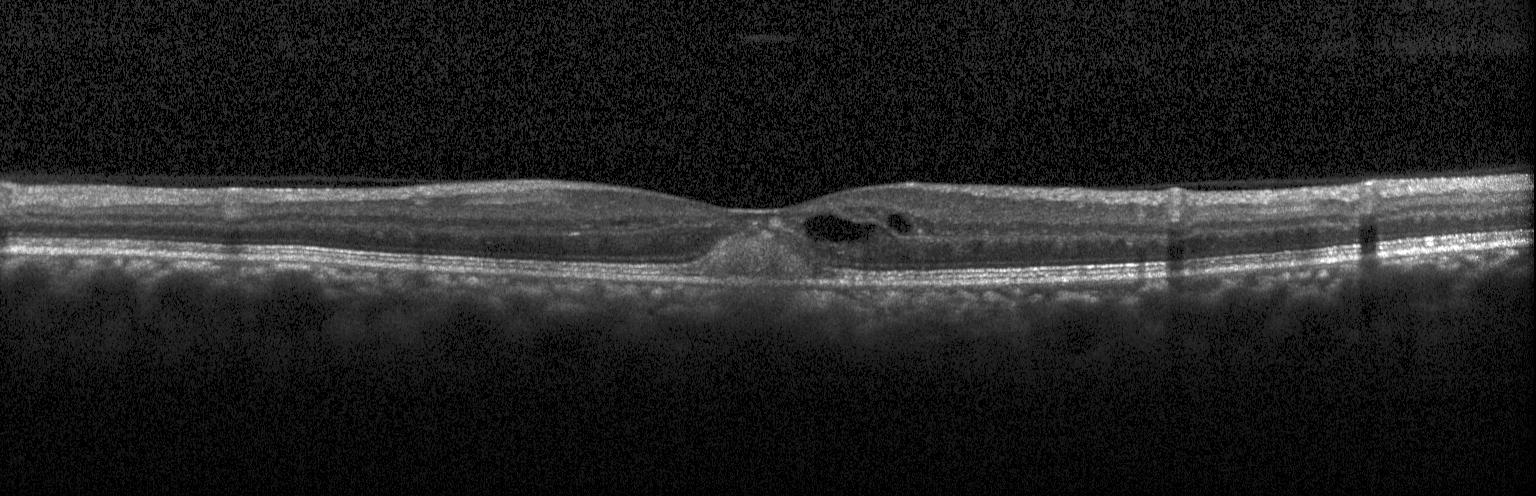

Spectral-domain OCT. OCT B-scan.
This B-scan demonstrates choroidal neovascularization (CNV).